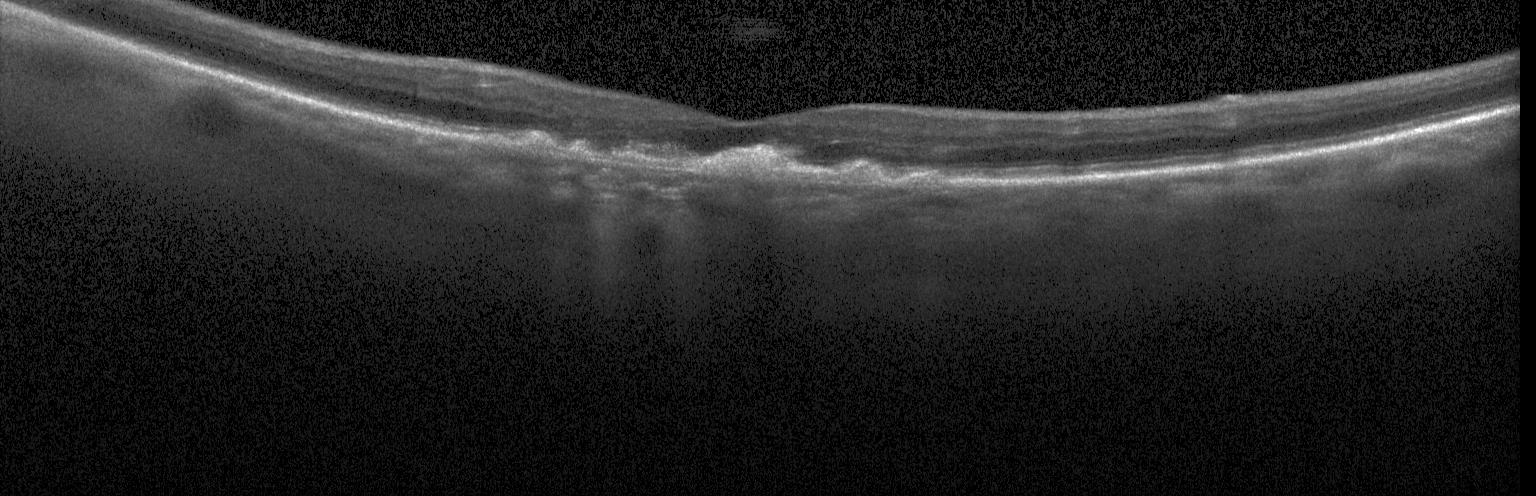 OCT B-scan — The scan shows a choroidal neovascular membrane.